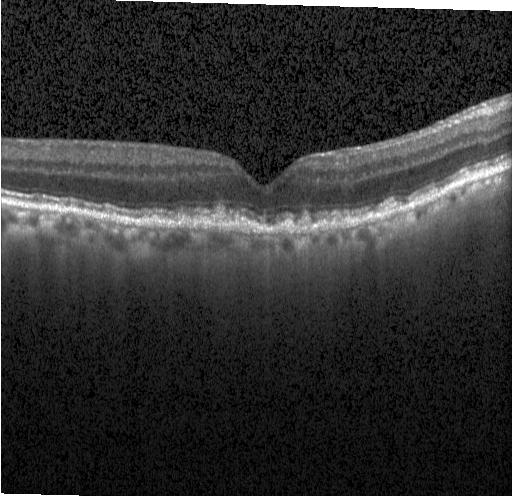

Through the macula · retinal OCT cross-section · Heidelberg Spectralis OCT system
Multiple drusen.